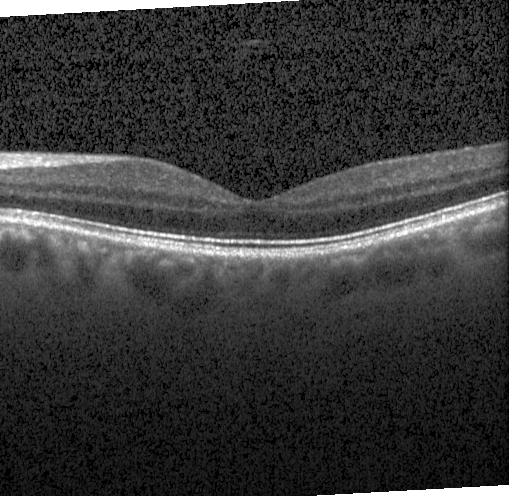

Diagnosis: neither choroidal neovascularization, diabetic macular edema, nor drusen.